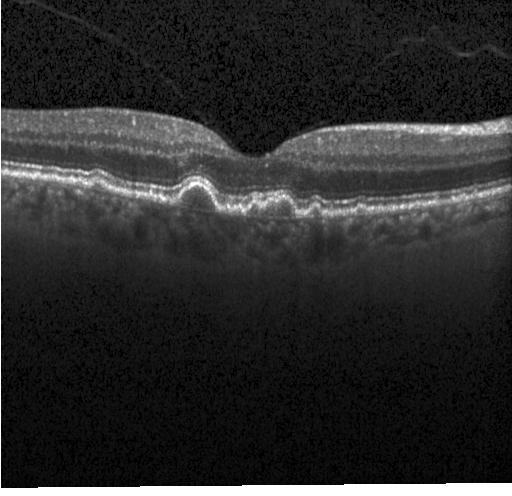 Dx: sub-RPE drusenoid deposits.